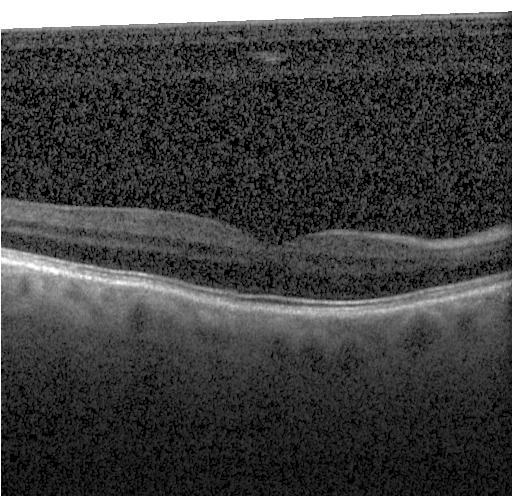 OCT line scan.
Assessment: no evidence of CNV, DME, or drusen.